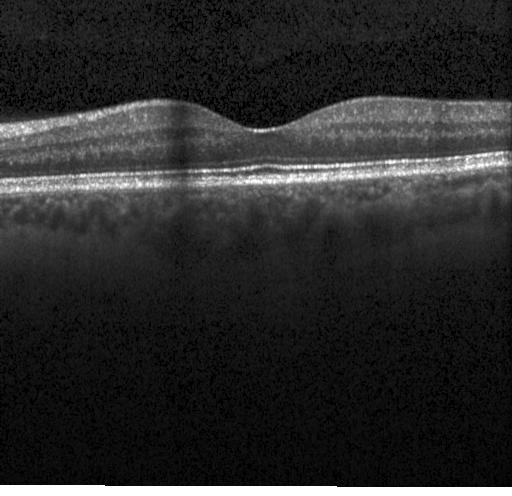

Impression: no choroidal neovascularization, diabetic macular edema, or drusen.